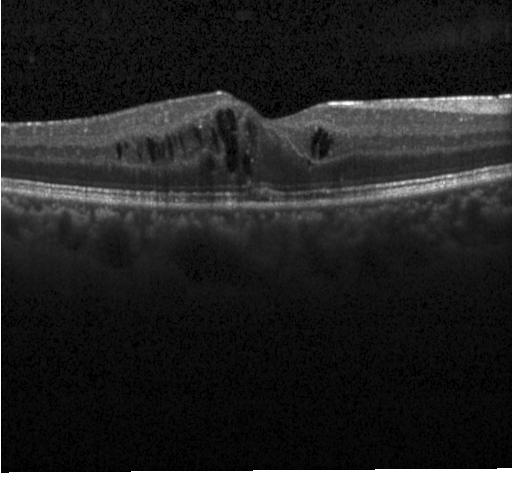

Retinal OCT B-scan, instrument: Heidelberg Spectralis, fovea-centered. Dx: DME.